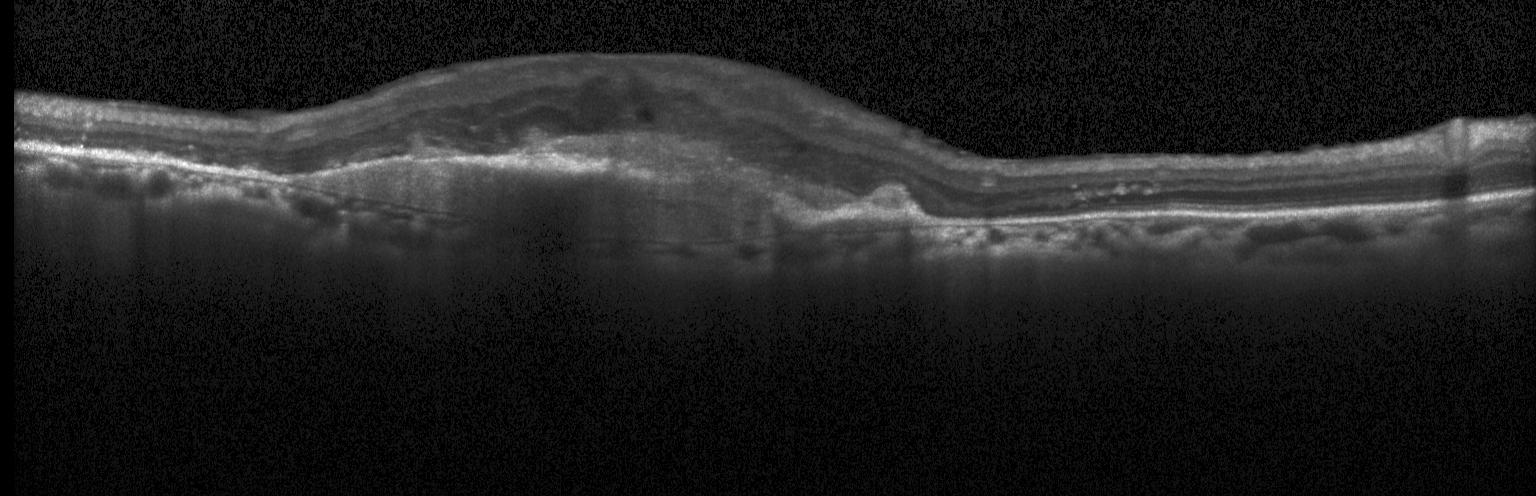

Spectral-domain OCT, OCT B-scan, Heidelberg Spectralis OCT system.
Choroidal neovascularization (CNV).